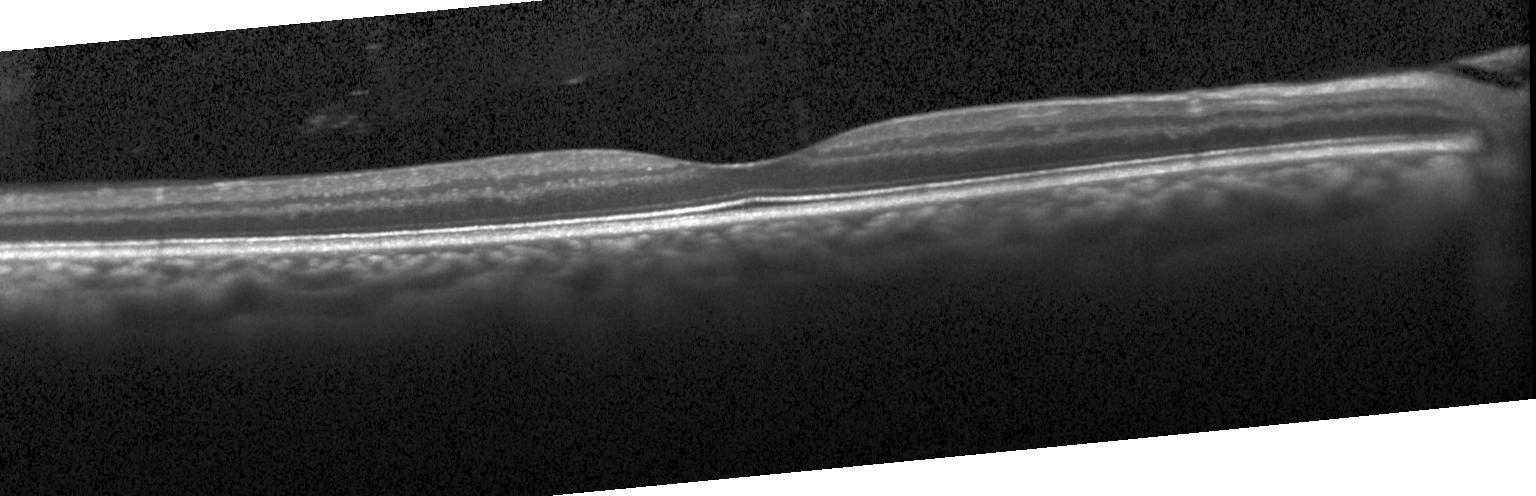
Retinal OCT B-scan.
OCT finding: no choroidal neovascularization, no diabetic macular edema, and no drusen.